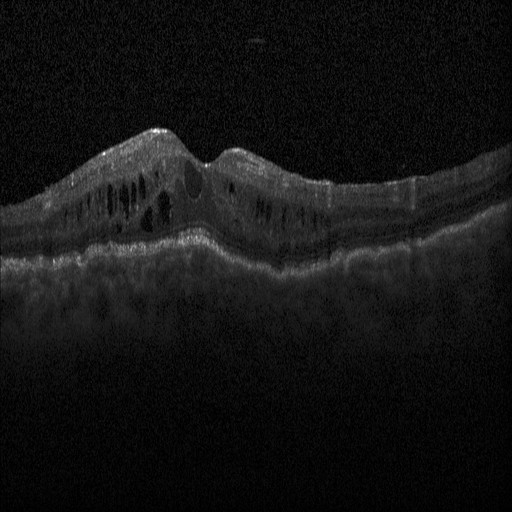

Horizontal scan through the fovea. Instrument: Heidelberg Spectralis. Retinal OCT cross-section — Impression: diabetic macular edema.